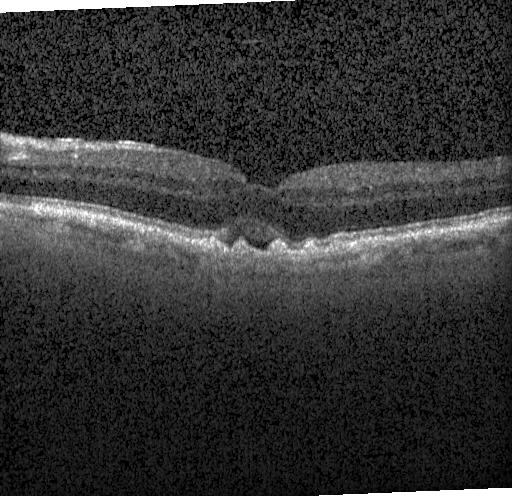 Spectral-domain OCT; retinal OCT B-scan; macular scan; instrument: Heidelberg Spectralis — Diagnosis: a choroidal neovascular membrane.